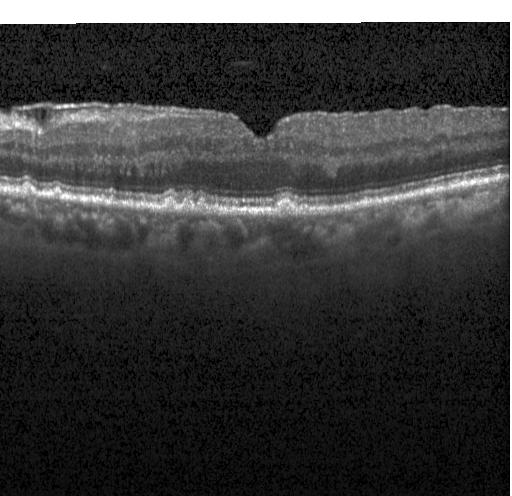 Impression: sub-RPE drusenoid deposits.